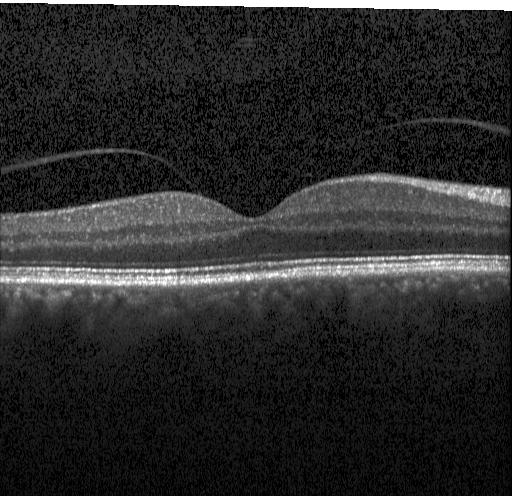

Fovea-centered. Optical coherence tomography B-scan — Finding: no evidence of choroidal neovascularization, diabetic macular edema, or drusen.